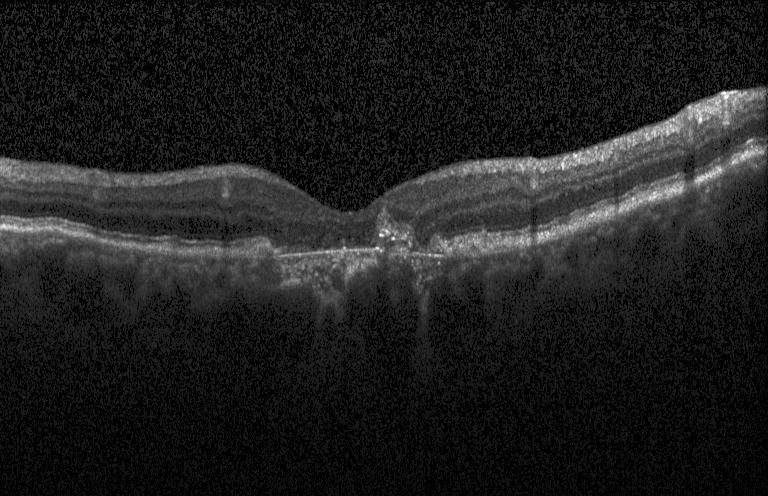
Retinal OCT B-scan.
Finding: a choroidal neovascular membrane.